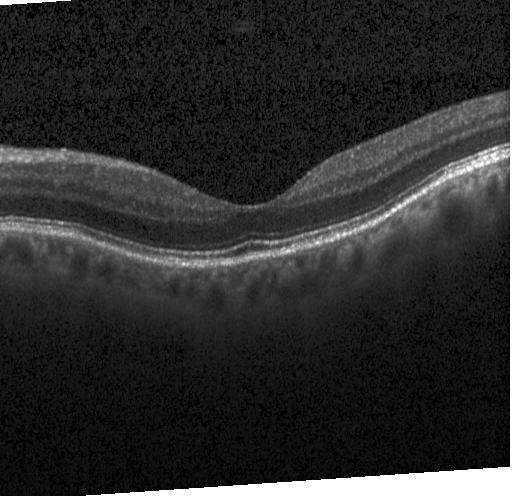

OCT B-scan, spectral-domain OCT, centered on the fovea. Impression: no CNV, no DME, and no drusen.